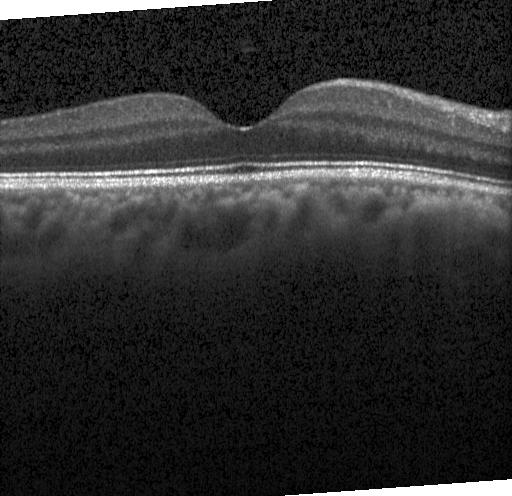

Assessment: neither CNV, DME, nor drusen.